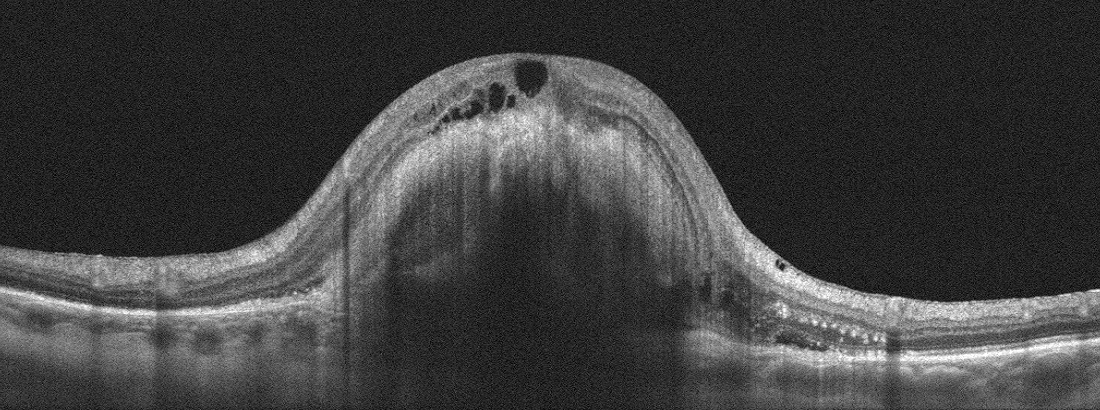 Impression: age-related macular degeneration (AMD).